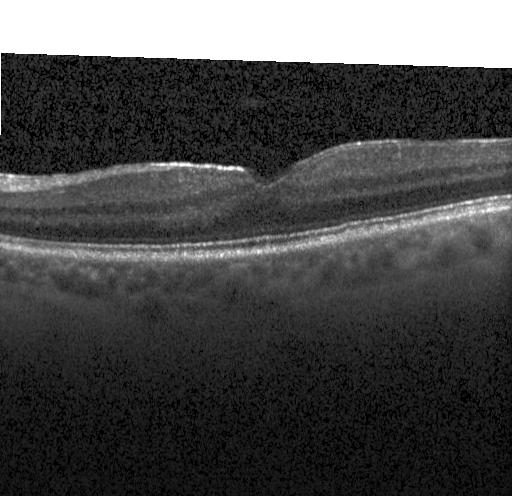 Finding: no choroidal neovascularization, diabetic macular edema, or drusen.